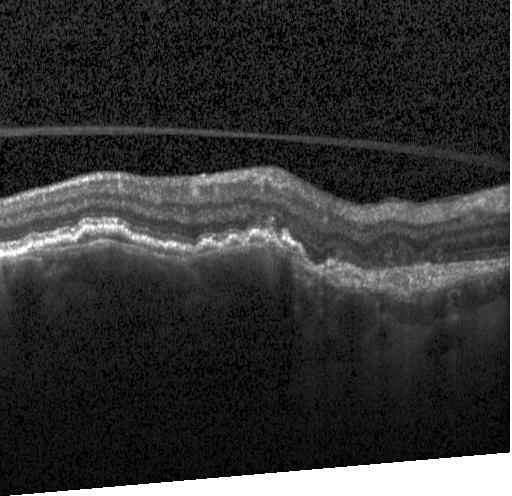
The scan shows a choroidal neovascular membrane.